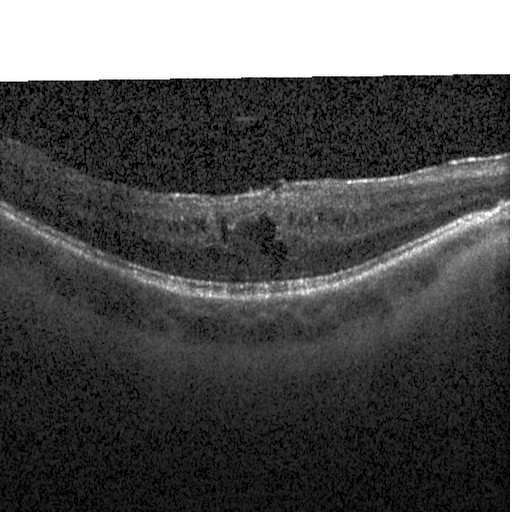

Optical coherence tomography scan, instrument: Heidelberg Spectralis — Diagnosis: diabetic macular edema.